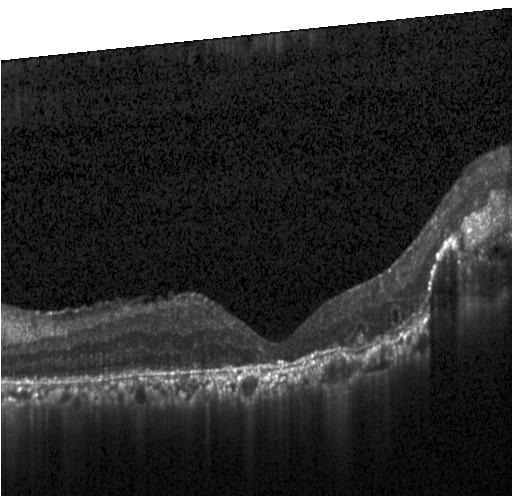
Through the macula. Acquired on a Heidelberg Spectralis. Retinal OCT B-scan — Impression: choroidal neovascularization.